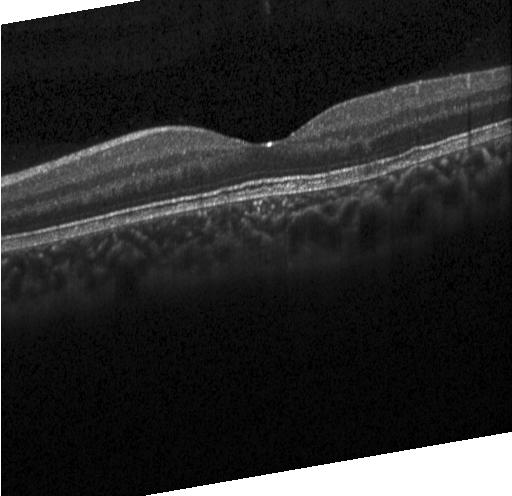

Horizontal scan through the fovea · retinal OCT B-scan · spectral-domain OCT · instrument: Heidelberg Spectralis — Macular OCT: neither choroidal neovascularization, diabetic macular edema, nor drusen.